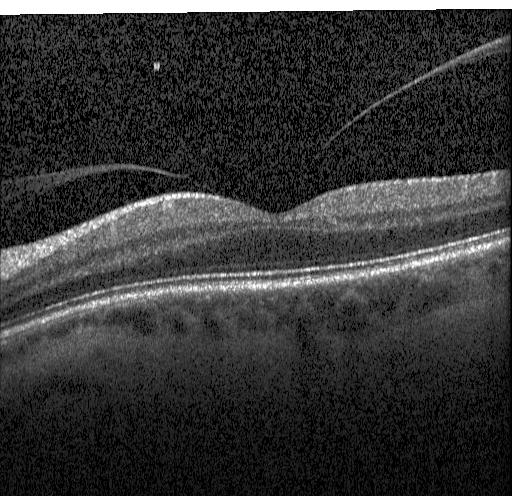

Retinal OCT cross-section.
Macular OCT: no CNV, DME, or drusen.